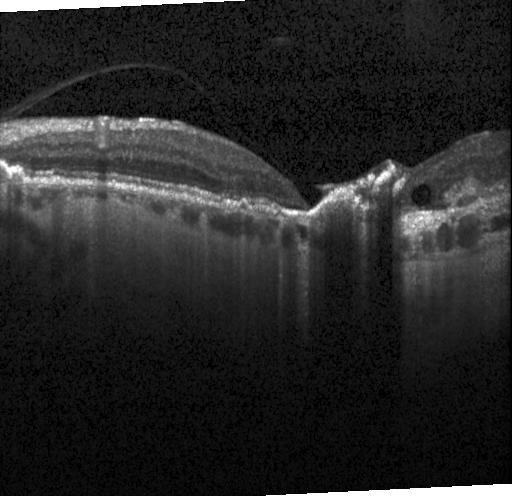

Diagnosis: choroidal neovascularization.